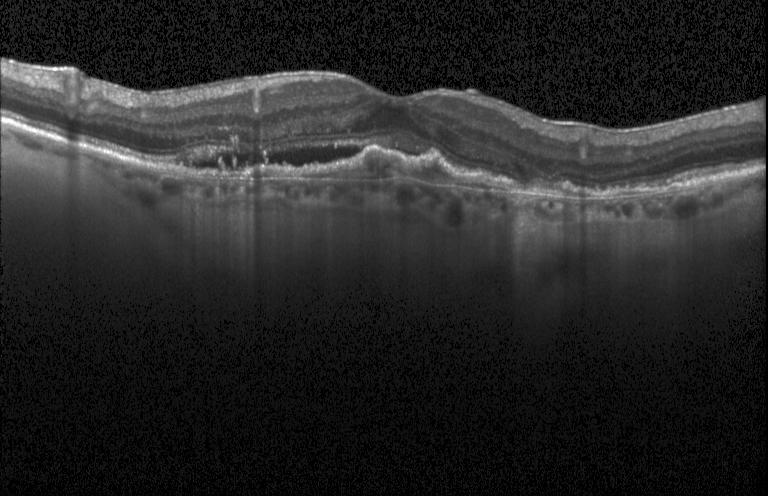

The scan shows choroidal neovascularization (CNV).